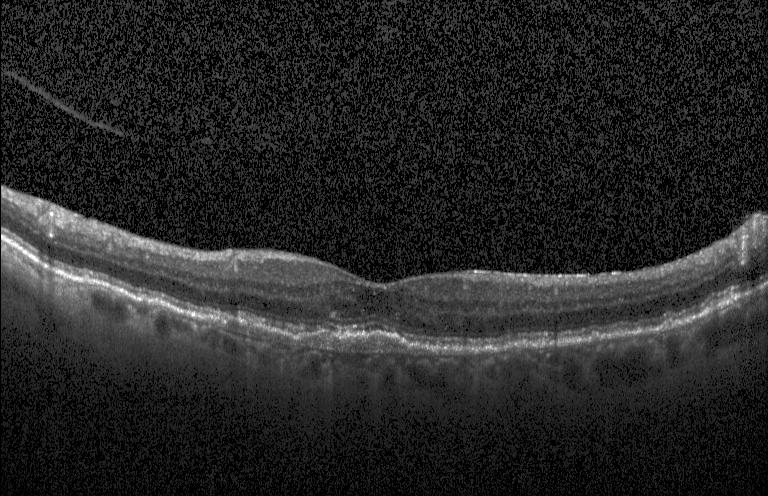 Spectral-domain optical coherence tomography. Optical coherence tomography scan. Heidelberg Spectralis OCT system — Diagnosis: CNV.